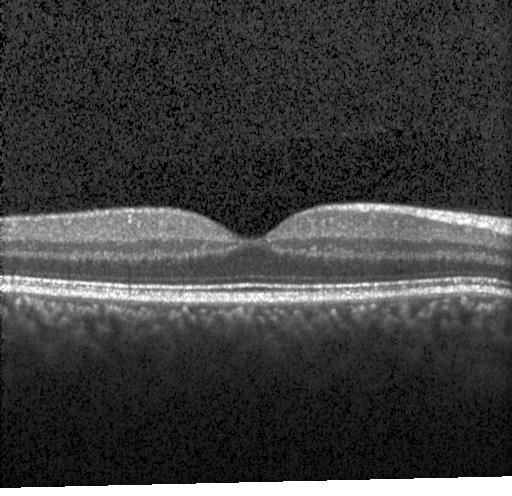 Through the macula · Heidelberg Spectralis OCT system · OCT B-scan · SD-OCT — This B-scan demonstrates no choroidal neovascularization, no diabetic macular edema, and no drusen.